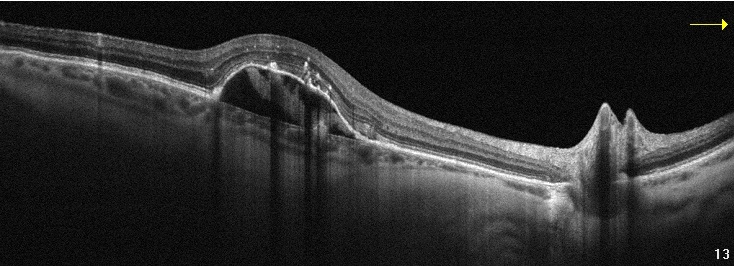 Optovue Avanti RTVue XR; OCT B-scan
Assessment: age-related macular degeneration.